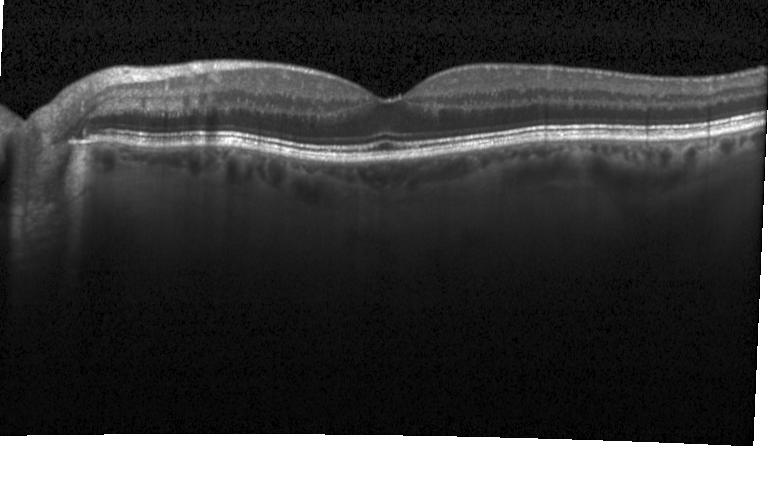

Heidelberg Spectralis; fovea-centered; SD-OCT; retinal OCT B-scan
Finding: no choroidal neovascularization, diabetic macular edema, or drusen.